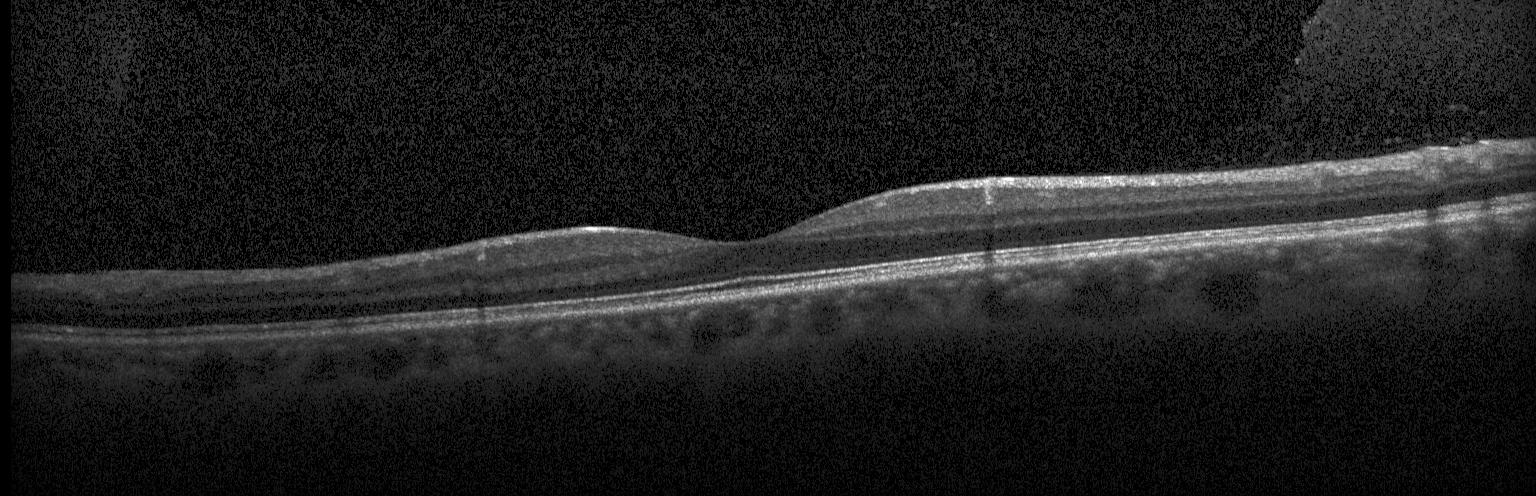 Assessment: no evidence of CNV, DME, or drusen.